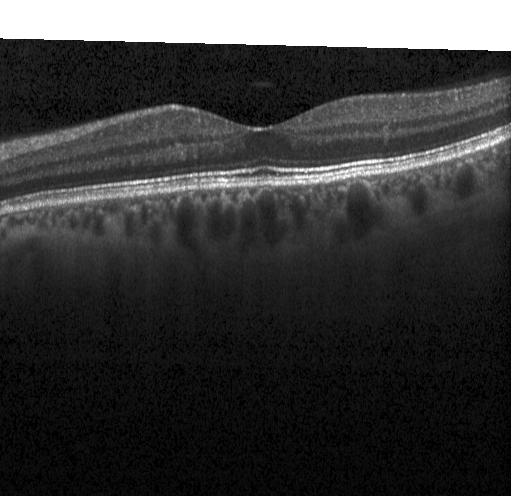
Finding: neither choroidal neovascularization, diabetic macular edema, nor drusen.